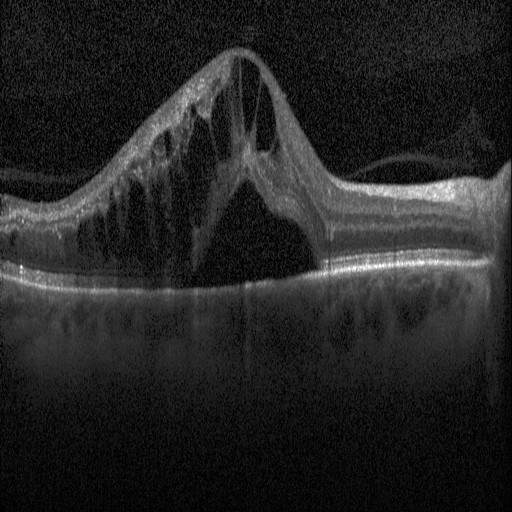

Spectral-domain OCT B-scan: diabetic macular edema.